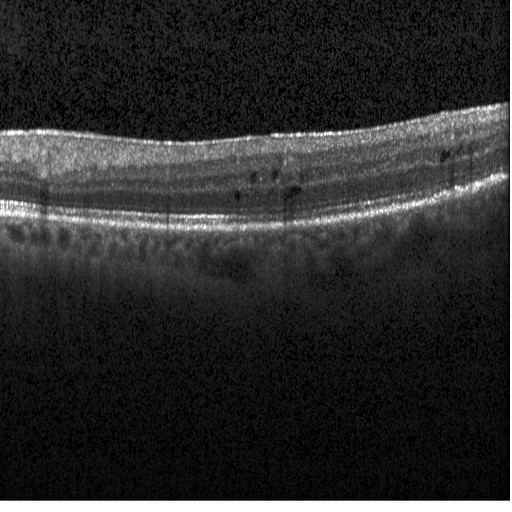

Optical coherence tomography scan · macular scan · spectral-domain optical coherence tomography
The scan shows diabetic macular edema.